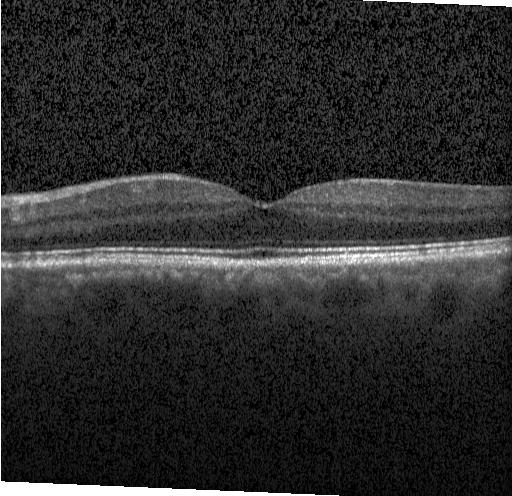

Heidelberg Spectralis; fovea-centered; OCT B-scan; SD-OCT.
Diagnosis: no evidence of choroidal neovascularization, diabetic macular edema, or drusen.